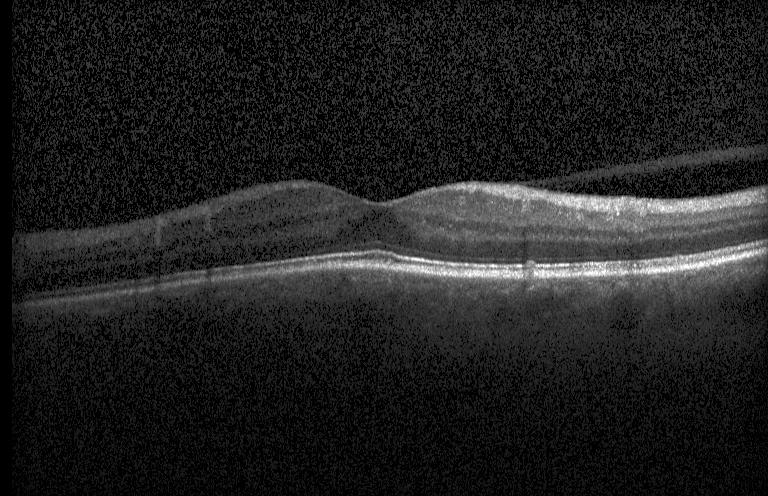 OCT finding: sub-RPE drusenoid deposits.